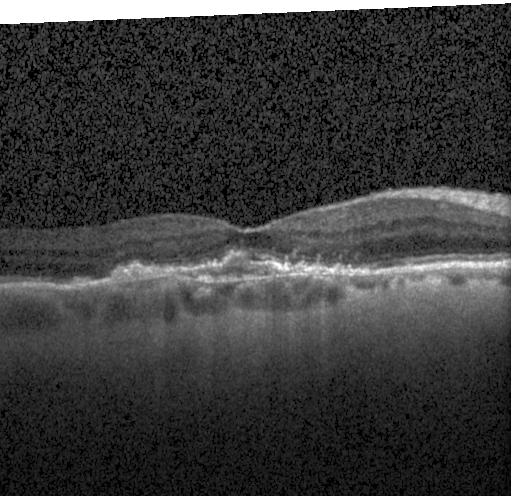

Horizontal scan through the fovea. Acquired on a Heidelberg Spectralis. Spectral-domain optical coherence tomography. Optical coherence tomography scan. The scan shows CNV.